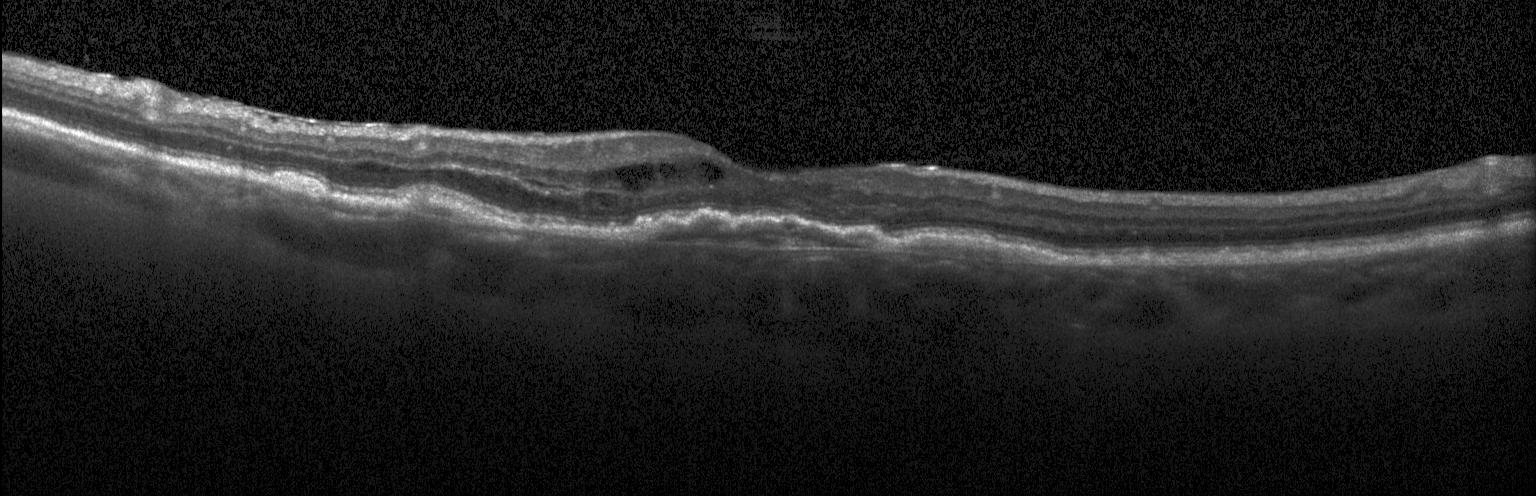

Finding: a choroidal neovascular membrane.